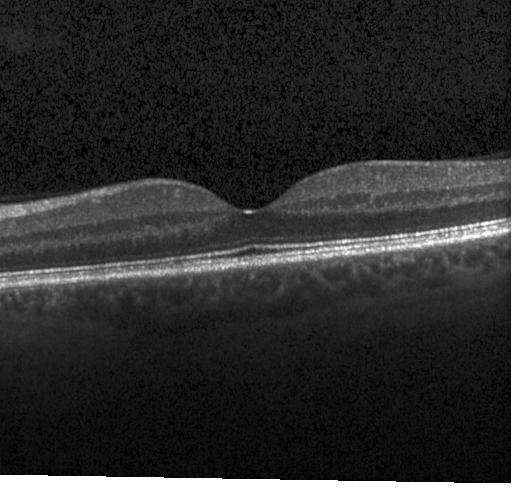

Instrument: Heidelberg Spectralis; macular scan; OCT line scan; spectral-domain OCT
Finding: neither choroidal neovascularization, diabetic macular edema, nor drusen.